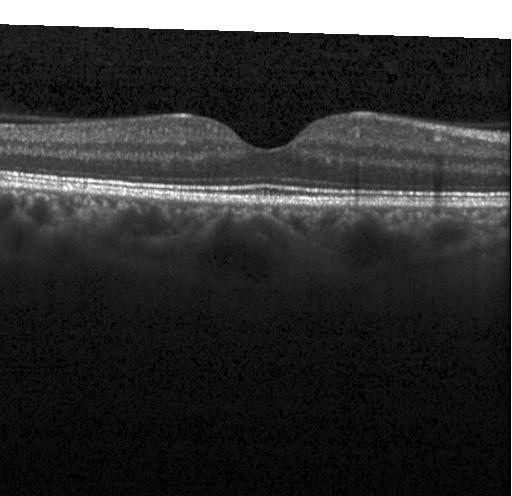 Spectral-domain OCT, retinal OCT B-scan, acquired on a Heidelberg Spectralis, fovea-centered.
Finding: no choroidal neovascularization, diabetic macular edema, or drusen.